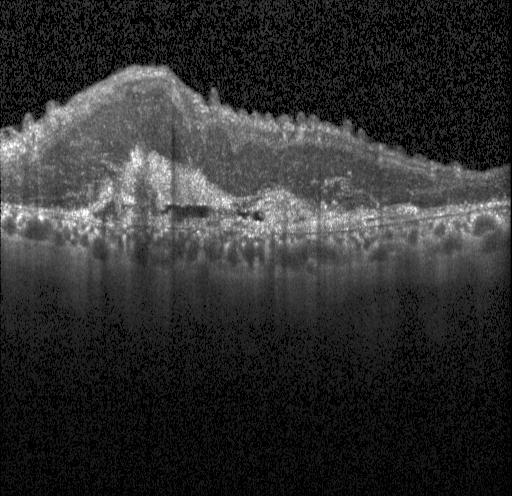

Retinal OCT cross-section showing a choroidal neovascular membrane.